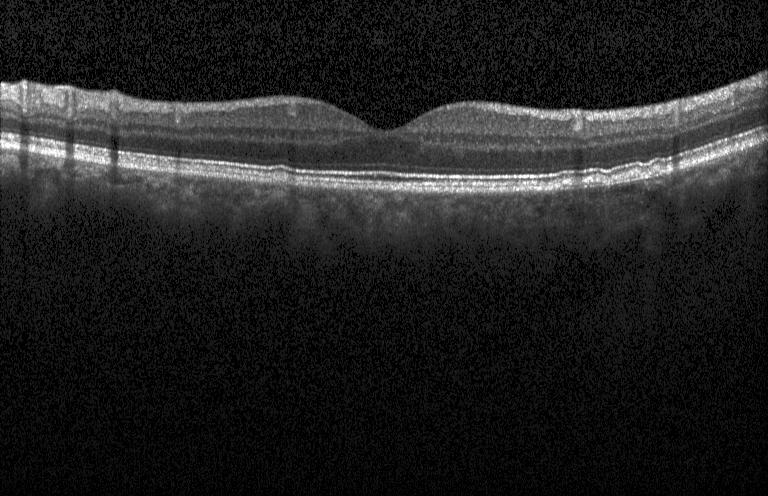 Retinal OCT cross-section showing drusen.